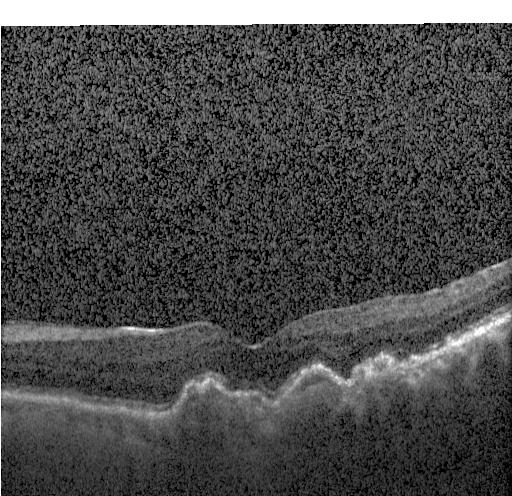 Retinal OCT cross-section showing a choroidal neovascular membrane.